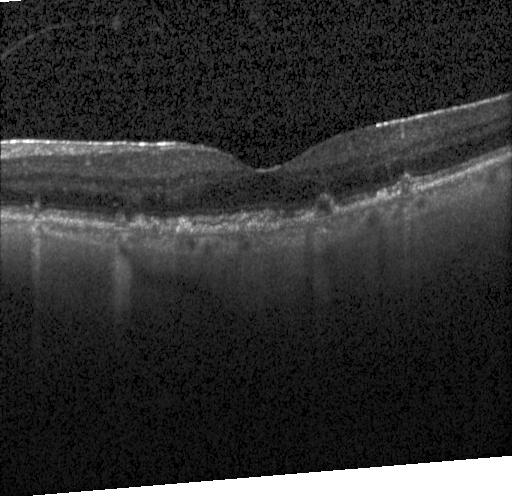
Finding: multiple drusen.